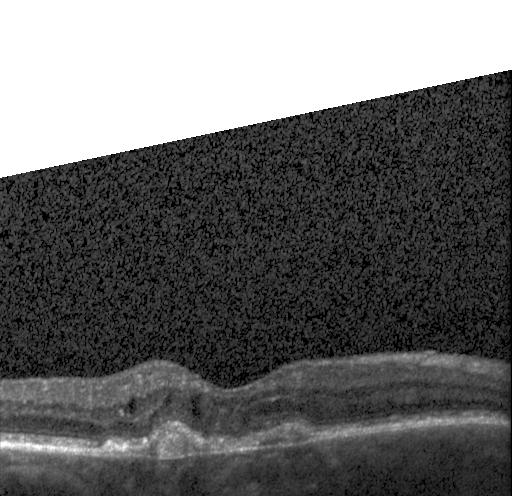 OCT B-scan showing CNV.